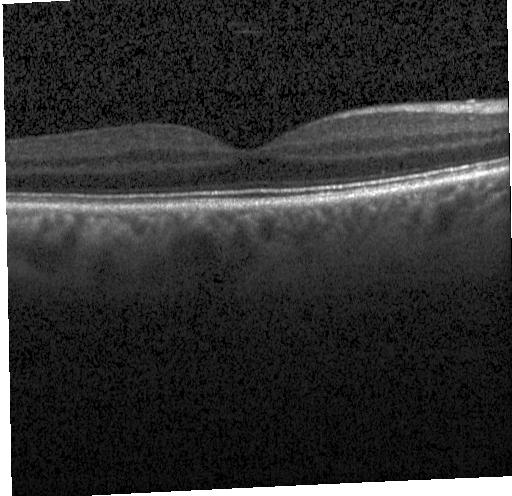
Dx: no choroidal neovascularization, no diabetic macular edema, and no drusen.